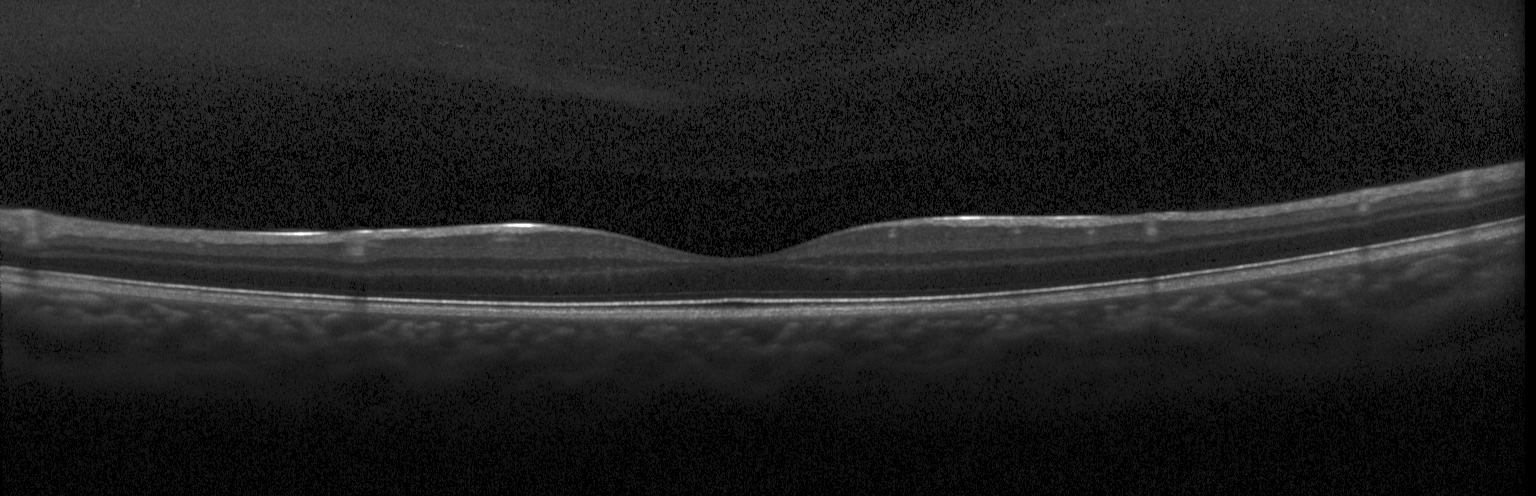 Optical coherence tomography B-scan. Impression: neither choroidal neovascularization, diabetic macular edema, nor drusen.